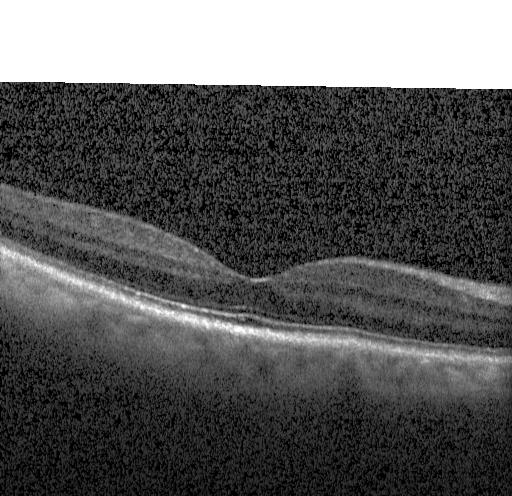

Heidelberg Spectralis · fovea-centered · SD-OCT · retinal OCT B-scan. Macular OCT: neither choroidal neovascularization, diabetic macular edema, nor drusen.